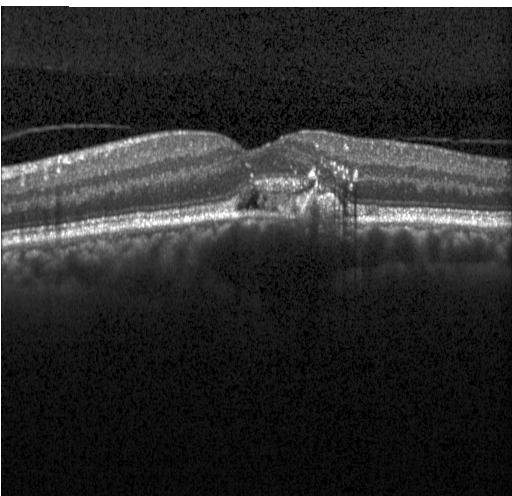
OCT B-scan showing choroidal neovascularization.